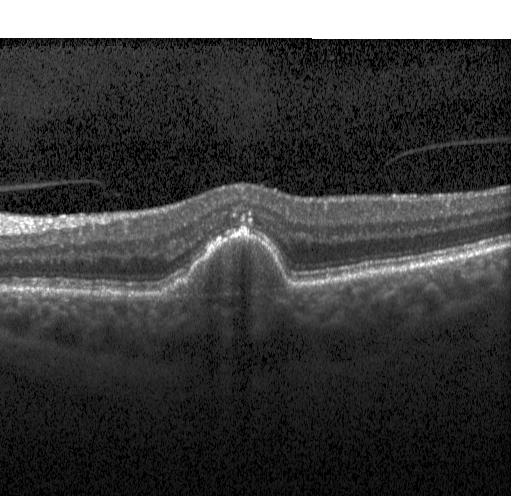

OCT line scan — Diagnosis: a choroidal neovascular membrane.